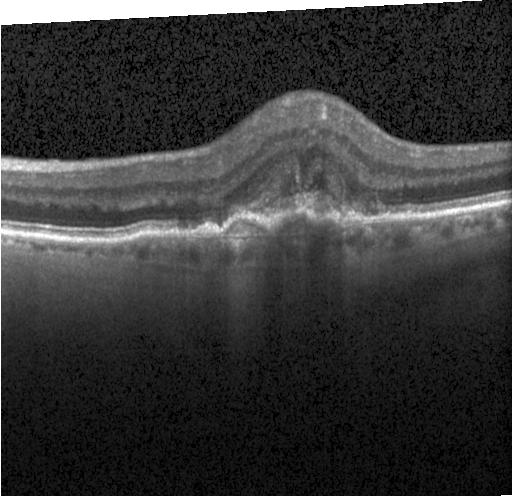
Dx: CNV.